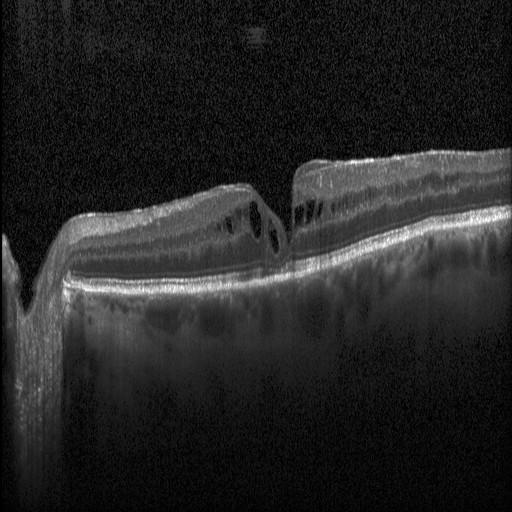

Fovea-centered. Retinal OCT B-scan. Heidelberg Spectralis. SD-OCT. Assessment: DME.